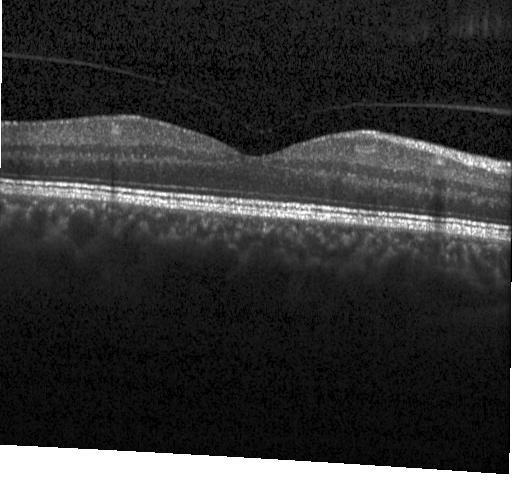 OCT scan showing no choroidal neovascularization, diabetic macular edema, or drusen.